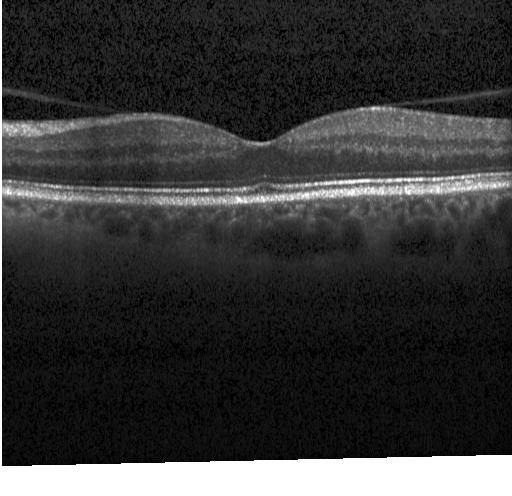

Spectral-domain OCT B-scan: no choroidal neovascularization, diabetic macular edema, or drusen.